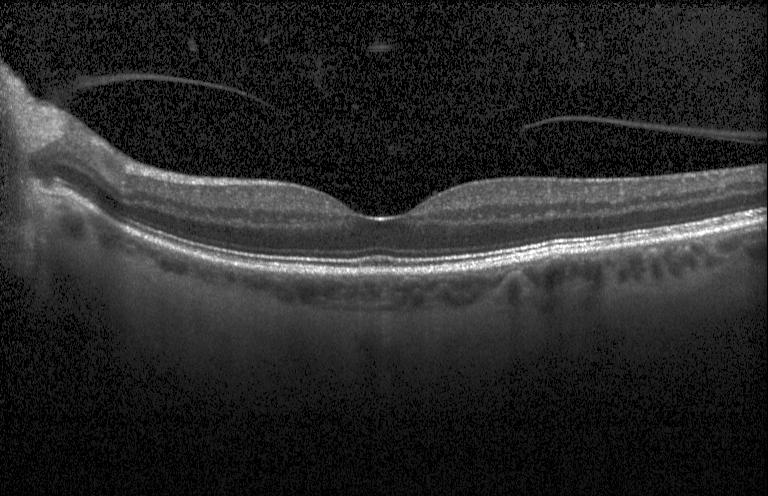
OCT line scan. Spectral-domain optical coherence tomography. Heidelberg Spectralis OCT system. Fovea-centered. Finding: no choroidal neovascularization, diabetic macular edema, or drusen.